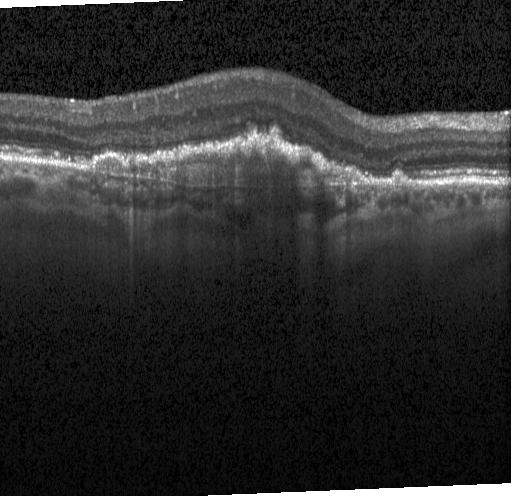

Heidelberg Spectralis, retinal OCT B-scan.
OCT finding: CNV.